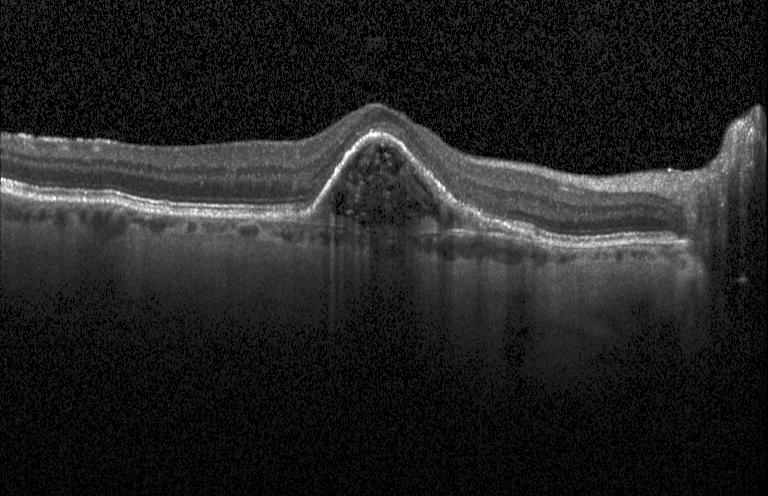

Heidelberg Spectralis OCT system · macular scan · retinal OCT B-scan · spectral-domain optical coherence tomography. Choroidal neovascularization (CNV).